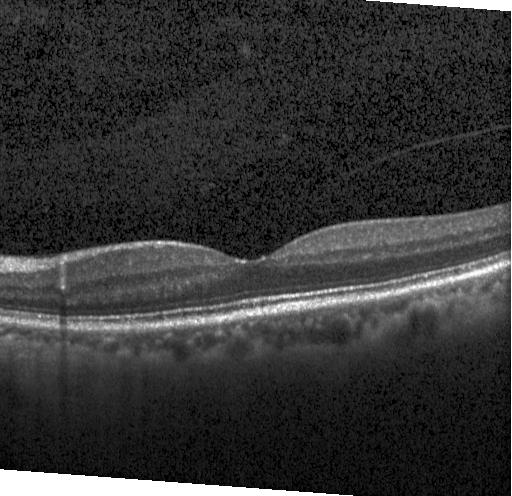

OCT line scan
Diagnosis: no choroidal neovascularization, diabetic macular edema, or drusen.